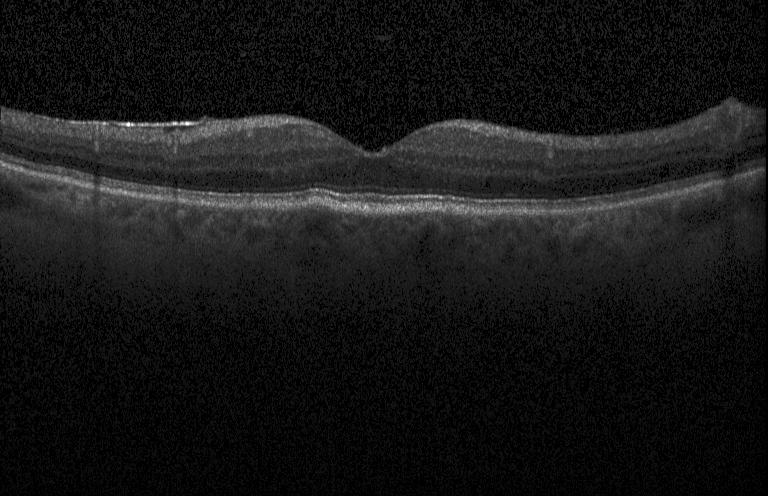
Optical coherence tomography scan
Finding: drusen.